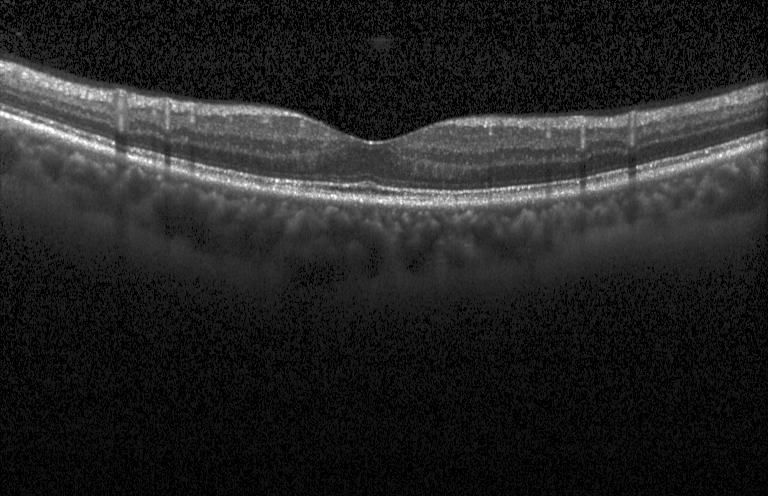

Optical coherence tomography B-scan; Heidelberg Spectralis.
Finding: neither choroidal neovascularization, diabetic macular edema, nor drusen.